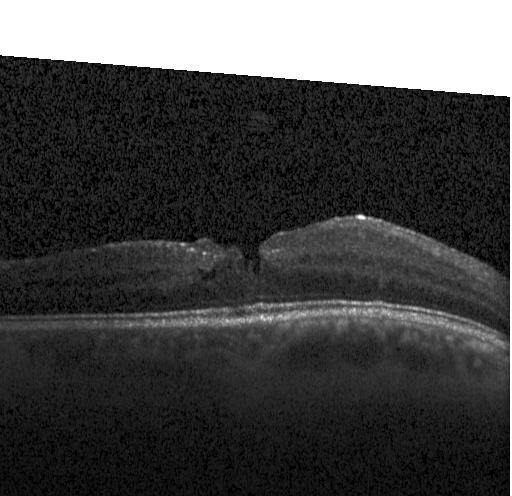

Retinal OCT B-scan; acquired on a Heidelberg Spectralis
Assessment: DME.